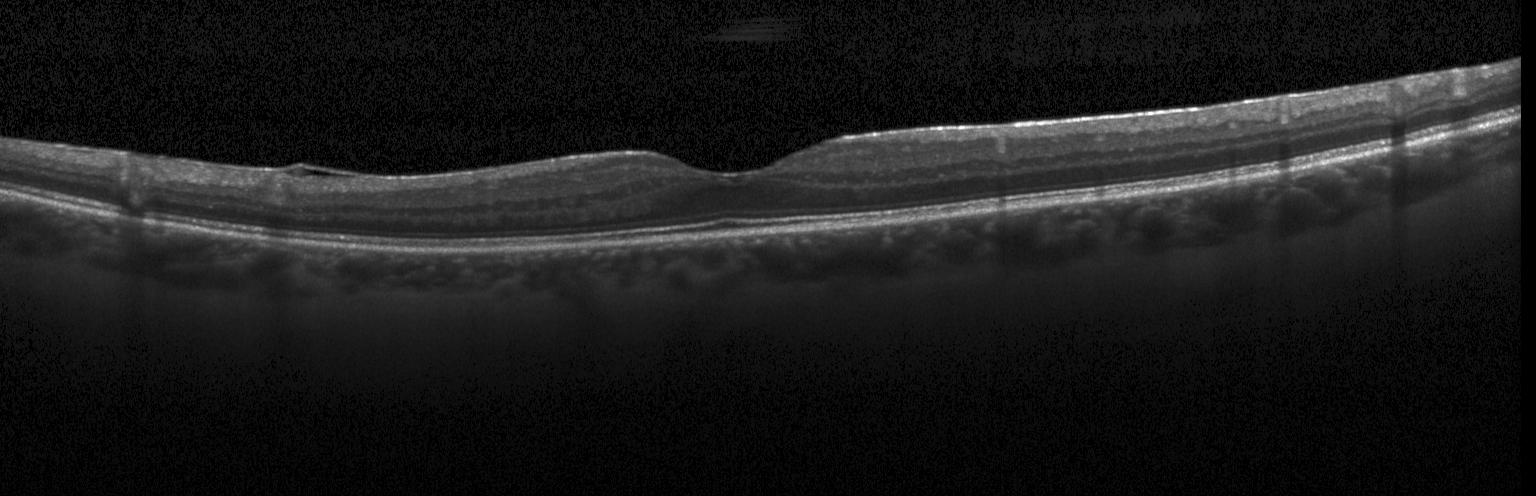
Heidelberg Spectralis · optical coherence tomography B-scan · horizontal scan through the fovea. Assessment: neither choroidal neovascularization, diabetic macular edema, nor drusen.